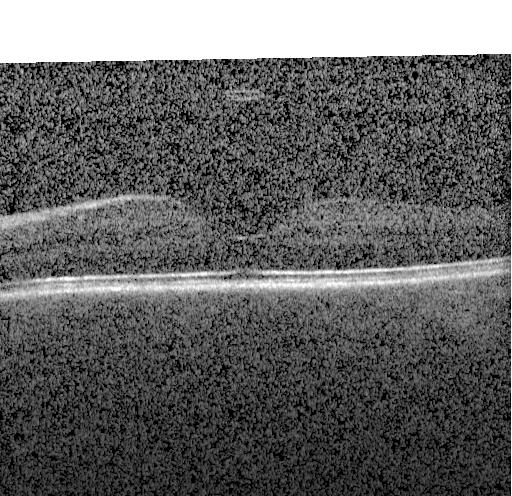

Finding: no evidence of choroidal neovascularization, diabetic macular edema, or drusen.